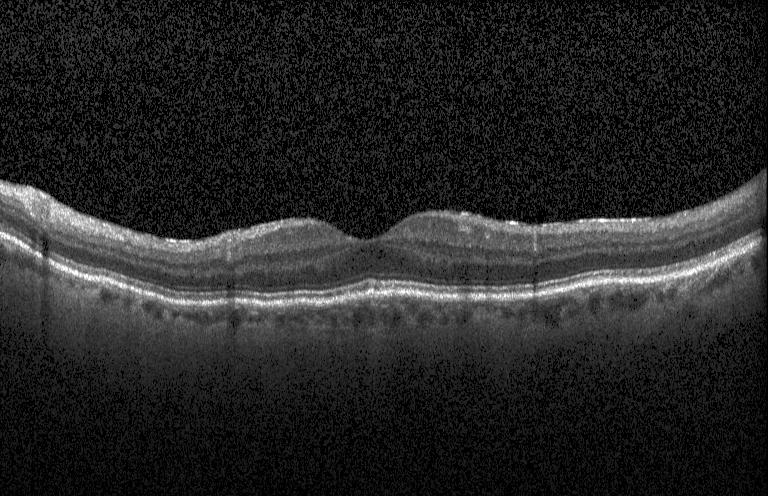

No CNV, DME, or drusen.